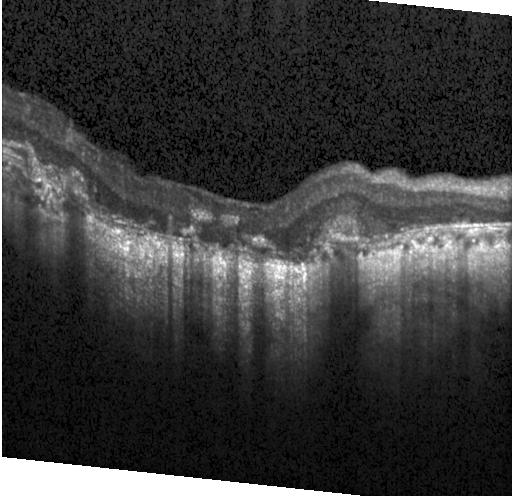
Diagnosis: a choroidal neovascular membrane.